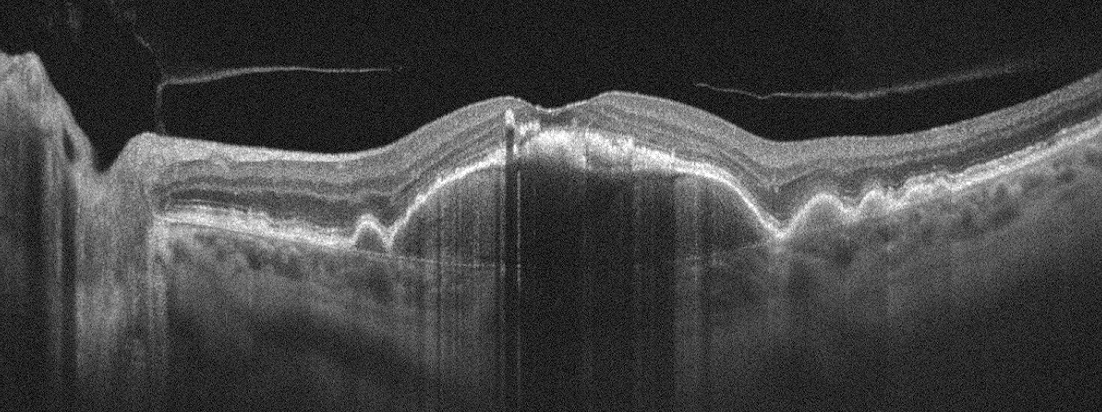
Dx: age-related macular degeneration (AMD).